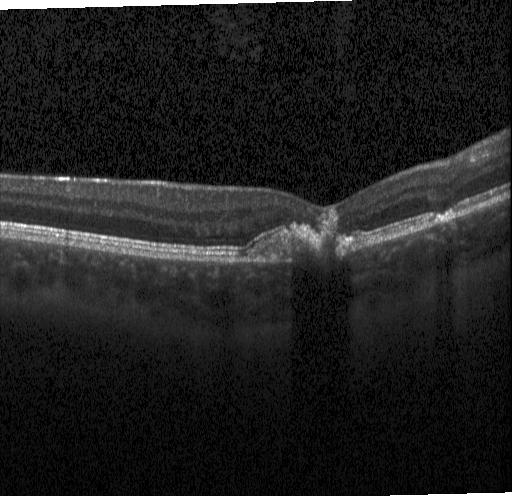
OCT B-scan
Diagnosis: a choroidal neovascular membrane.